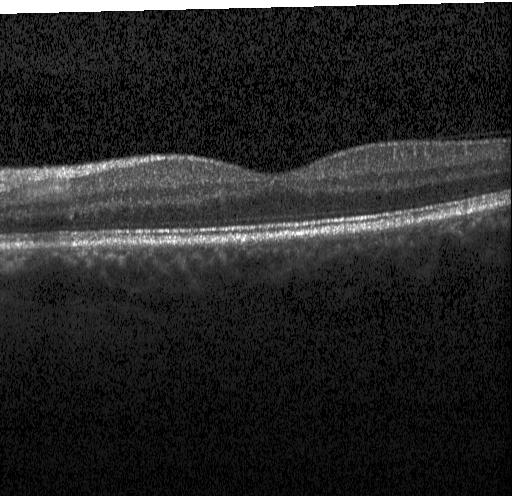 Spectral-domain OCT, instrument: Heidelberg Spectralis, OCT B-scan.
Diagnosis: no choroidal neovascularization, diabetic macular edema, or drusen.